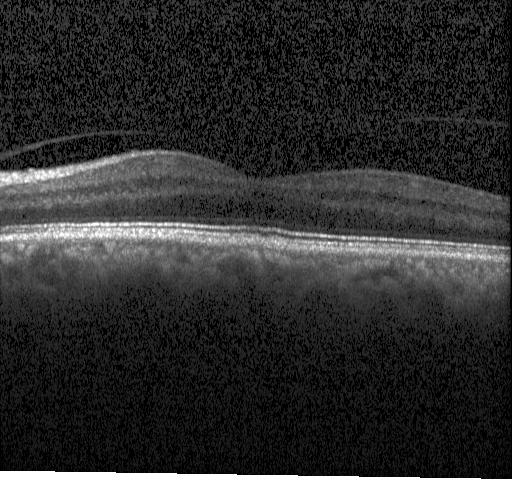 The scan shows neither choroidal neovascularization, diabetic macular edema, nor drusen.